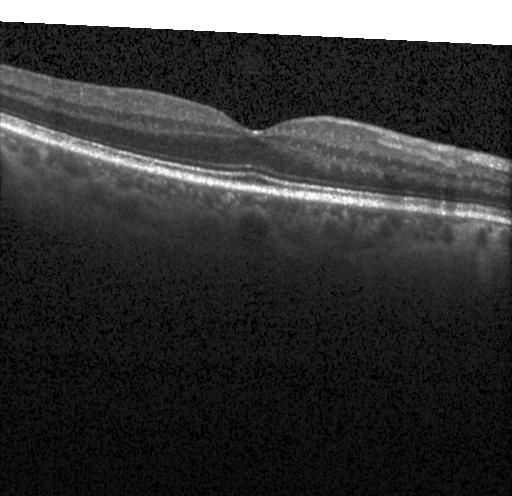 Finding: no evidence of CNV, DME, or drusen.